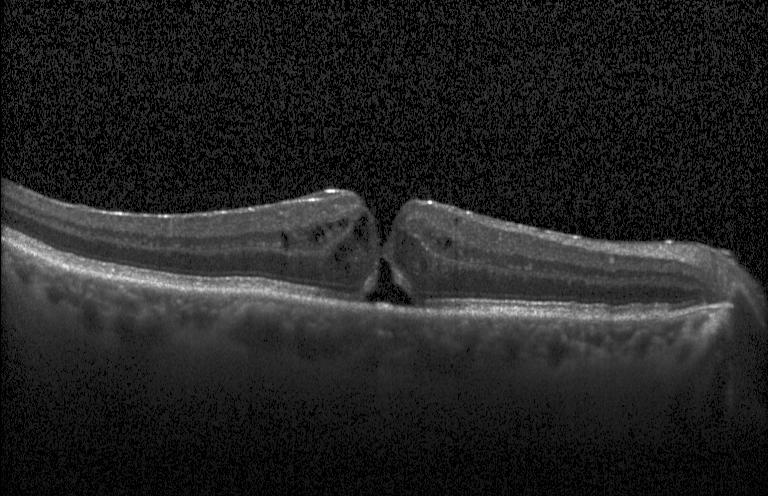
Retinal OCT cross-section. Acquired on a Heidelberg Spectralis. SD-OCT. Through the macula — The scan shows diabetic macular edema (DME).